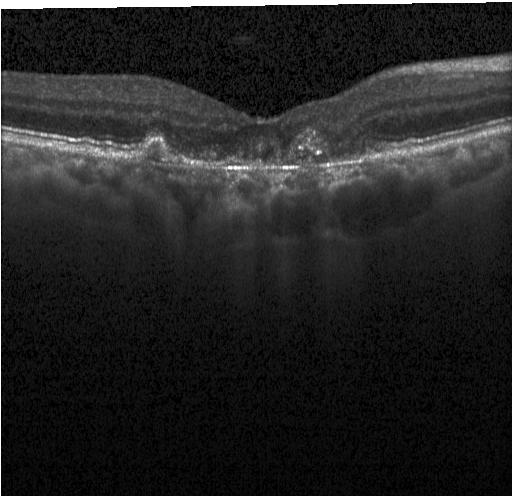 Macular OCT demonstrating a choroidal neovascular membrane.